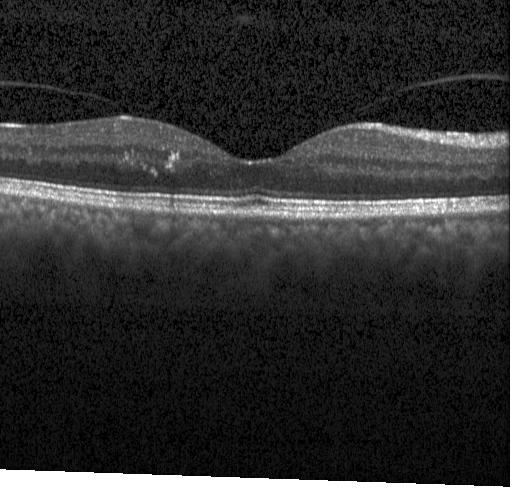 Optical coherence tomography B-scan, spectral-domain optical coherence tomography.
Dx: no choroidal neovascularization, no diabetic macular edema, and no drusen.